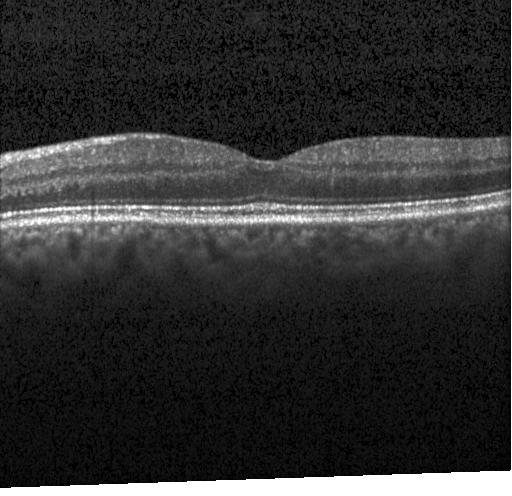

Macular OCT: no CNV, no DME, and no drusen.